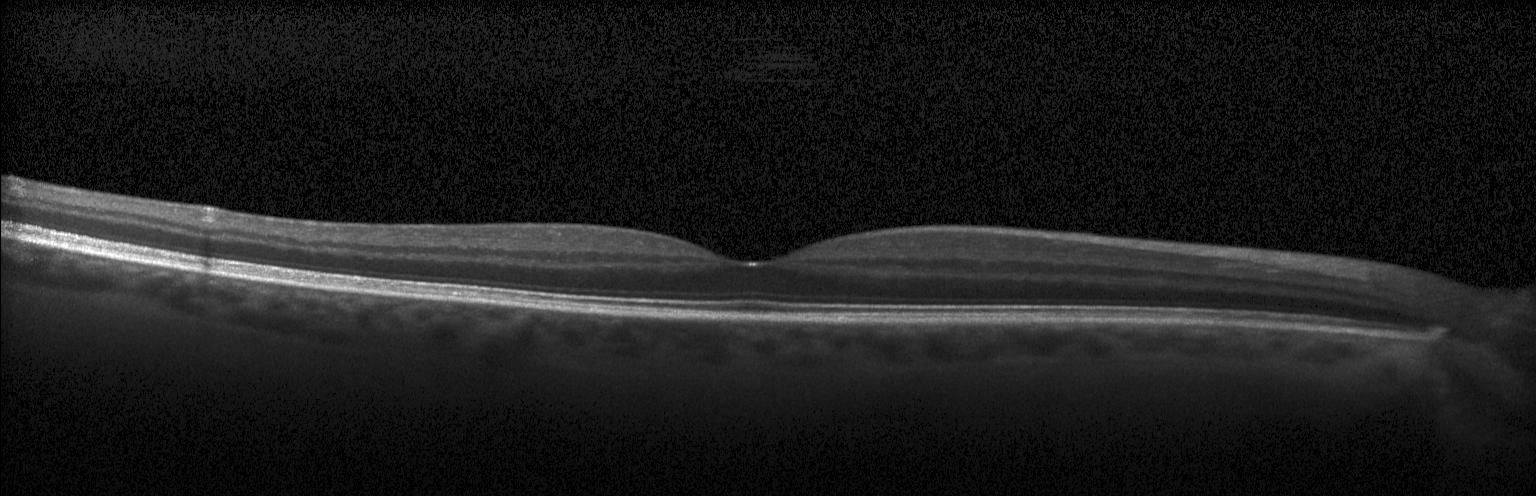 Spectral-domain OCT. Instrument: Heidelberg Spectralis. Optical coherence tomography B-scan. Macular scan — Finding: no CNV, DME, or drusen.